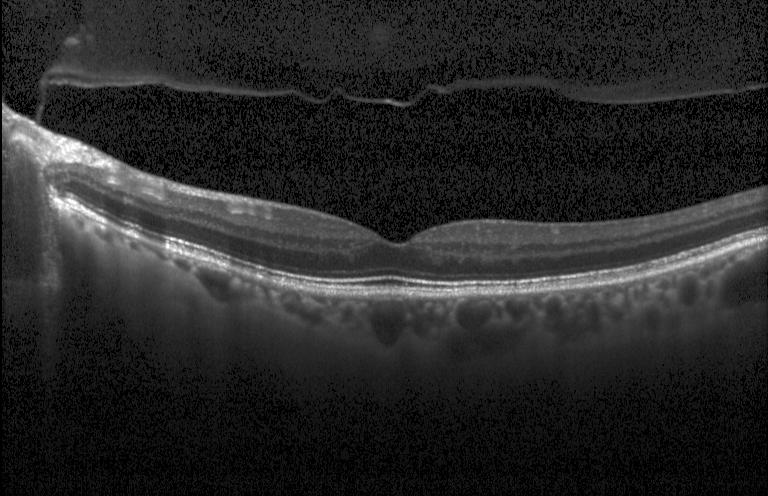 Dx: no CNV, DME, or drusen.